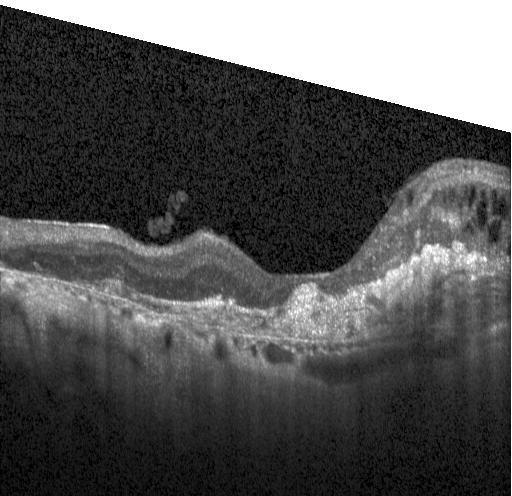

OCT B-scan showing a choroidal neovascular membrane.